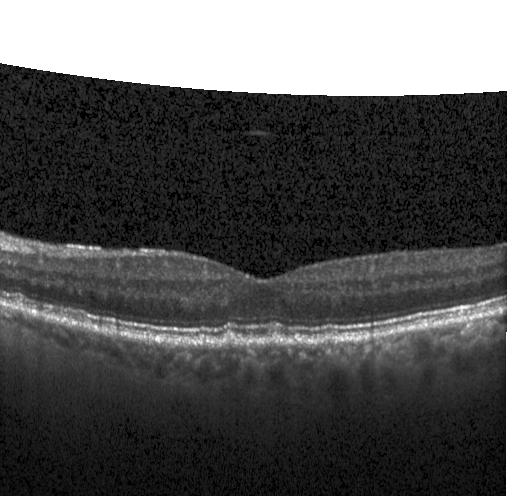

This B-scan demonstrates sub-RPE drusenoid deposits.